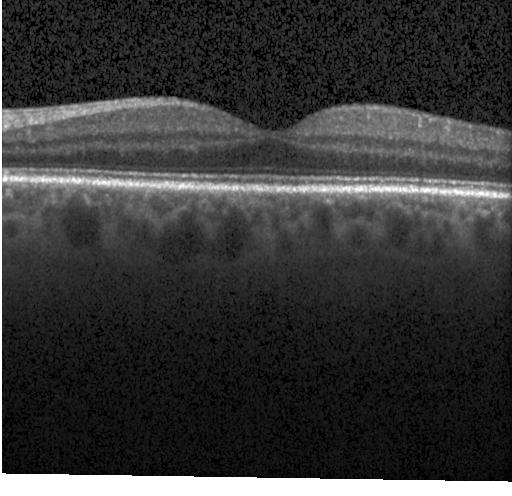

Horizontal scan through the fovea; SD-OCT; optical coherence tomography scan; Heidelberg Spectralis OCT system.
Assessment: no choroidal neovascularization, no diabetic macular edema, and no drusen.